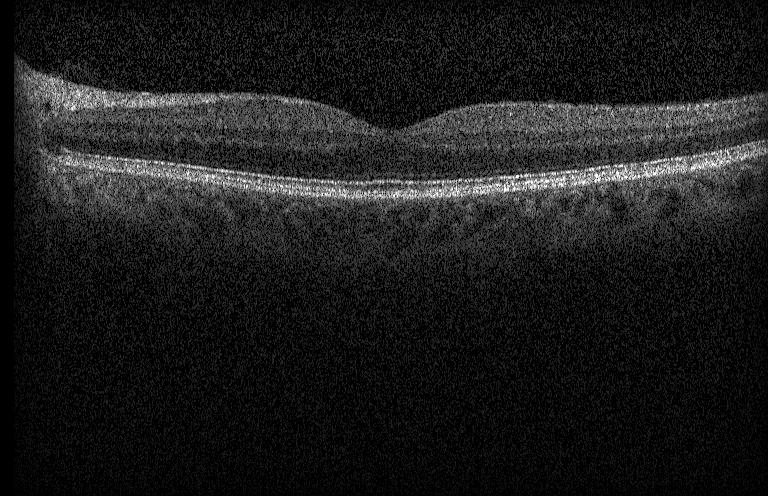
OCT line scan, centered on the fovea, spectral-domain optical coherence tomography — Dx: no evidence of choroidal neovascularization, diabetic macular edema, or drusen.